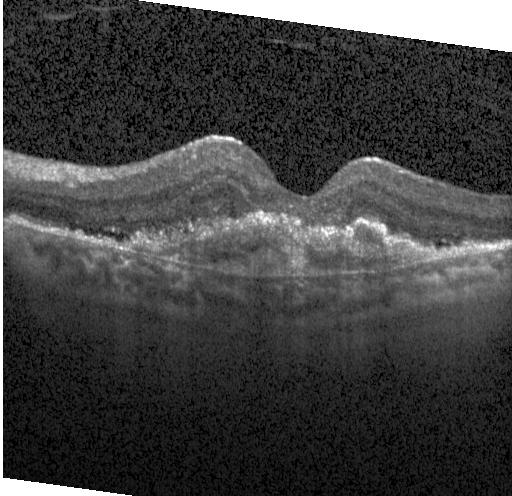
This B-scan demonstrates choroidal neovascularization.